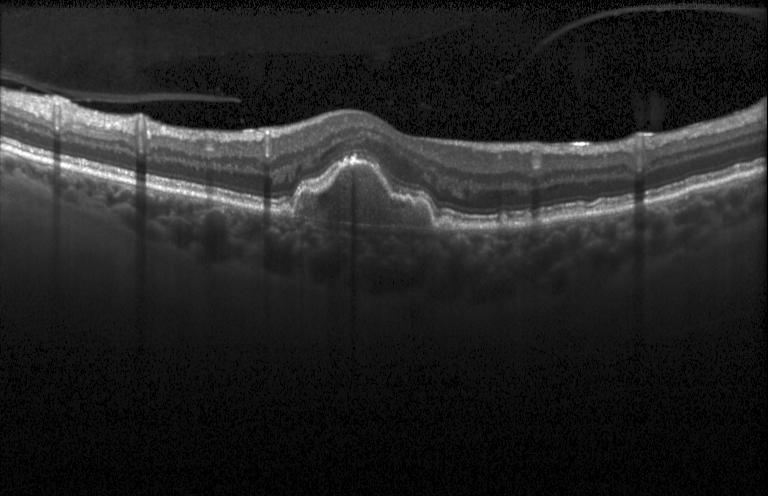 Heidelberg Spectralis; optical coherence tomography scan — Assessment: a choroidal neovascular membrane.